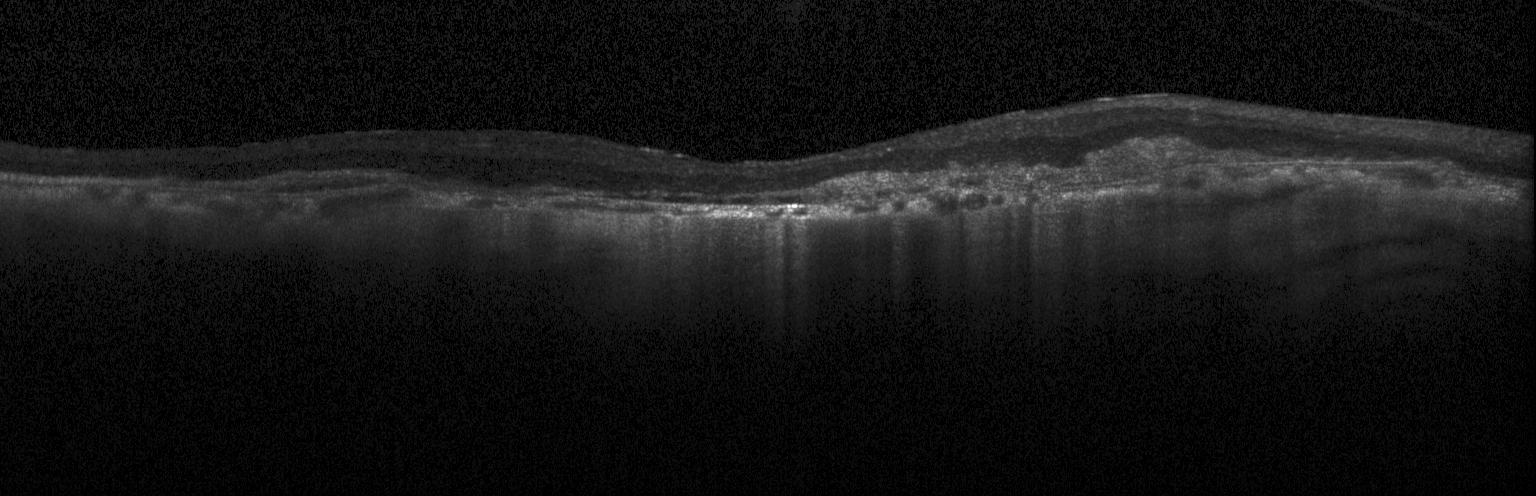
OCT B-scan. Macular OCT: choroidal neovascularization (CNV).